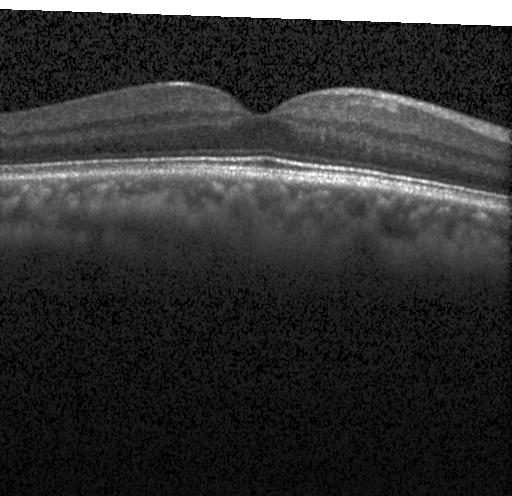 Dx: no choroidal neovascularization, diabetic macular edema, or drusen.